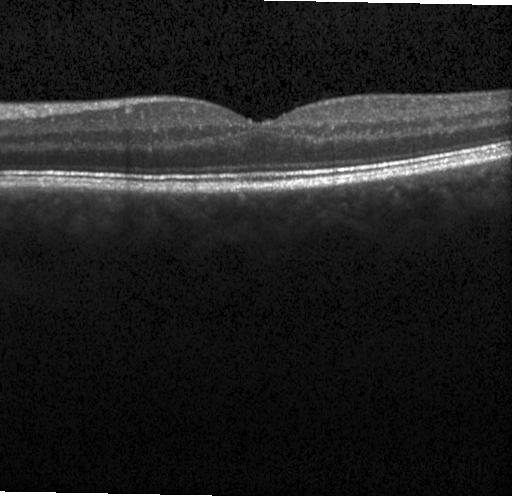 Retinal OCT cross-section — This B-scan demonstrates no CNV, no DME, and no drusen.